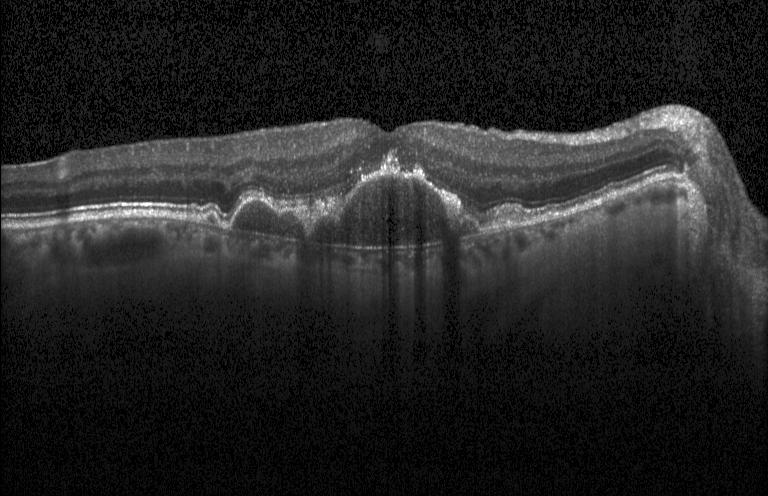

OCT scan showing a choroidal neovascular membrane.